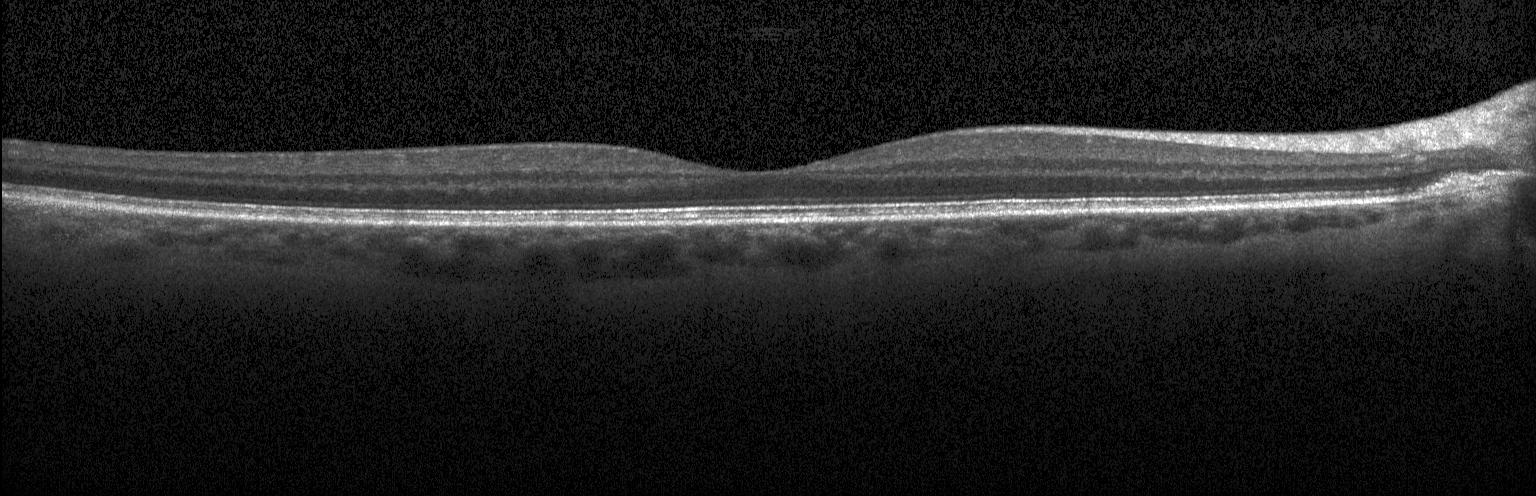 Fovea-centered · Heidelberg Spectralis · spectral-domain optical coherence tomography · OCT B-scan
Diagnosis: no evidence of choroidal neovascularization, diabetic macular edema, or drusen.